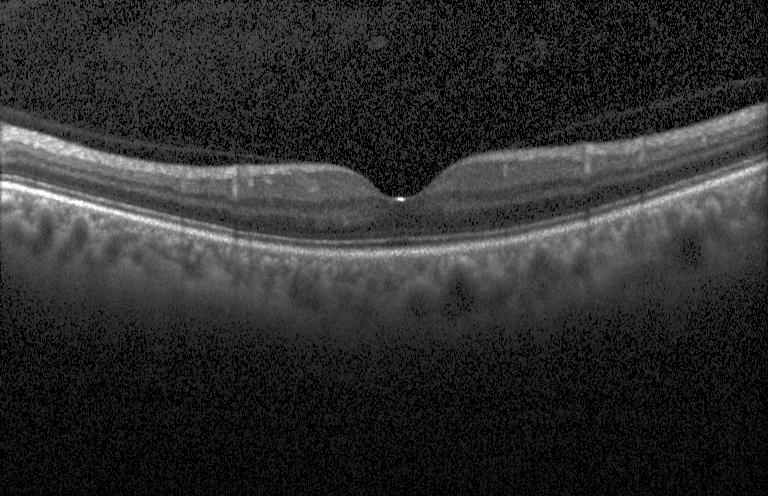
Finding: neither choroidal neovascularization, diabetic macular edema, nor drusen.